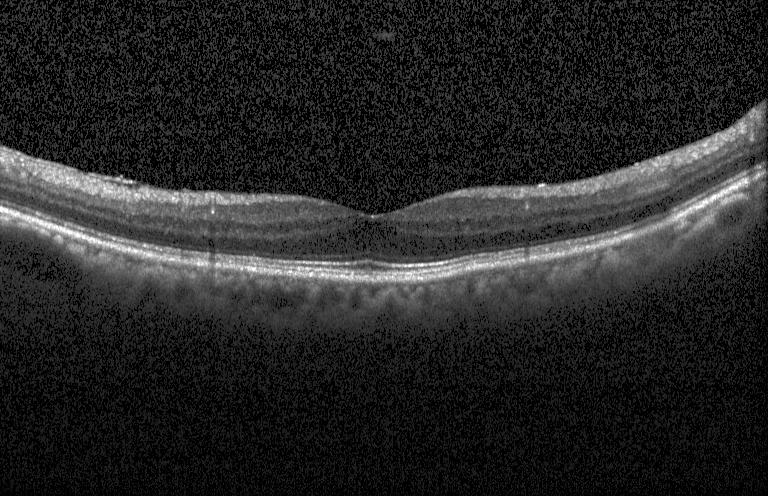 Diagnosis: no evidence of choroidal neovascularization, diabetic macular edema, or drusen.